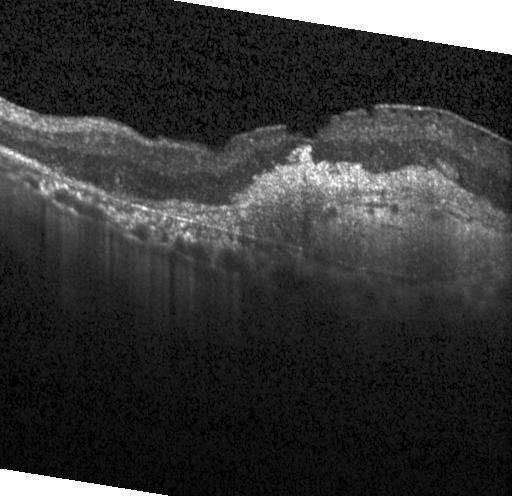 Retinal OCT cross-section · instrument: Heidelberg Spectralis · spectral-domain OCT — Impression: a choroidal neovascular membrane.